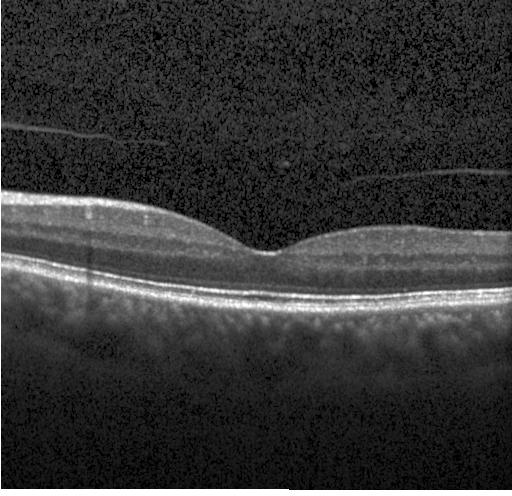 Optical coherence tomography B-scan. This B-scan demonstrates neither CNV, DME, nor drusen.